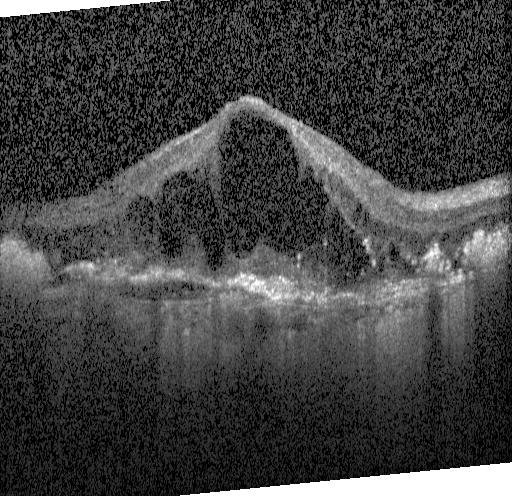 Spectral-domain OCT; retinal OCT B-scan — Finding: a choroidal neovascular membrane.